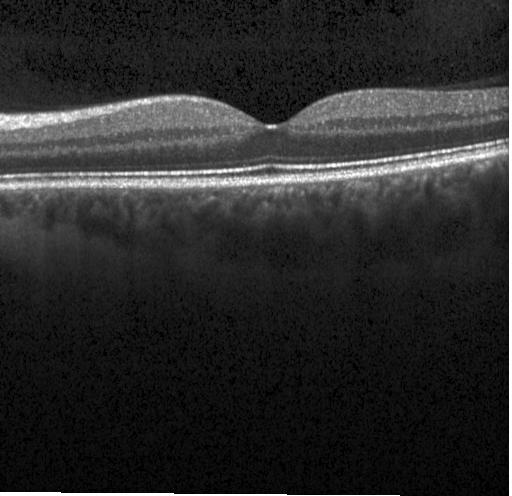

The scan shows no evidence of CNV, DME, or drusen.